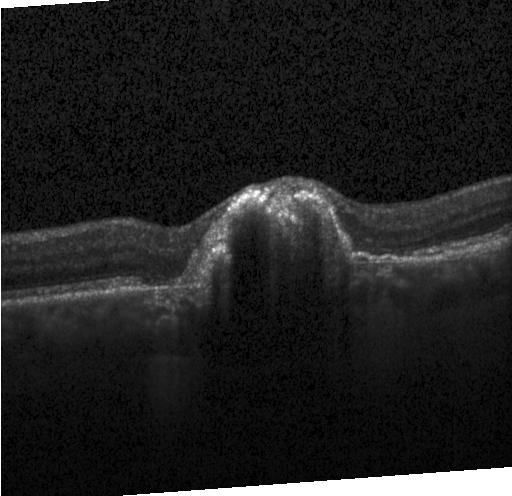 OCT line scan · acquired on a Heidelberg Spectralis.
Finding: choroidal neovascularization.